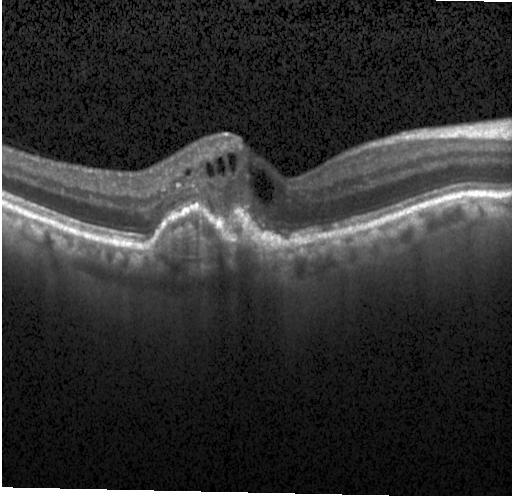
The scan shows choroidal neovascularization.